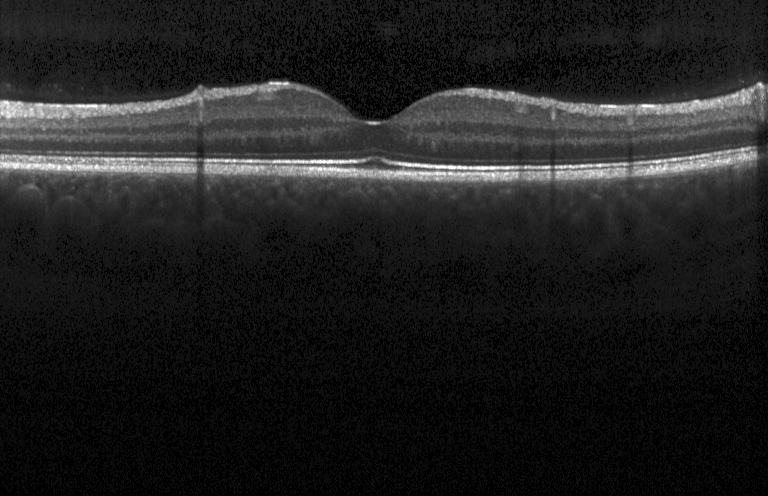 Finding: neither choroidal neovascularization, diabetic macular edema, nor drusen.